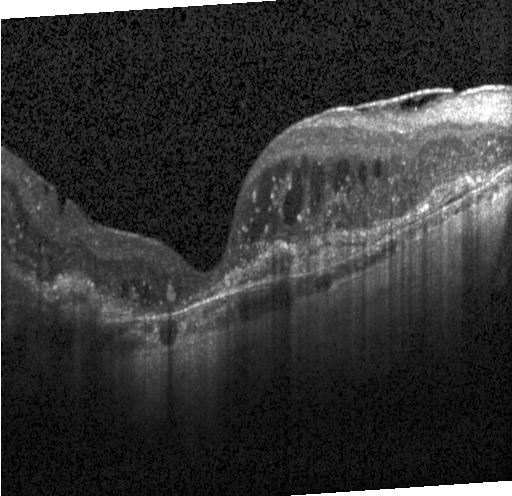

Instrument: Heidelberg Spectralis · optical coherence tomography scan · SD-OCT. CNV.